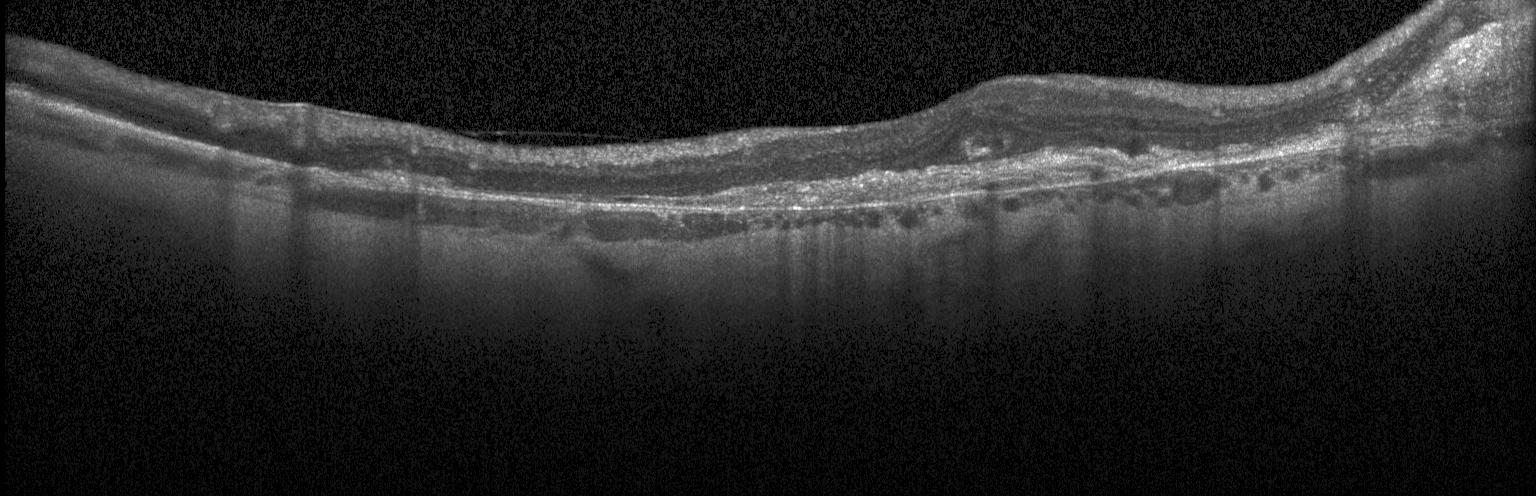 Retinal OCT B-scan. Horizontal scan through the fovea — Diagnosis: choroidal neovascularization.